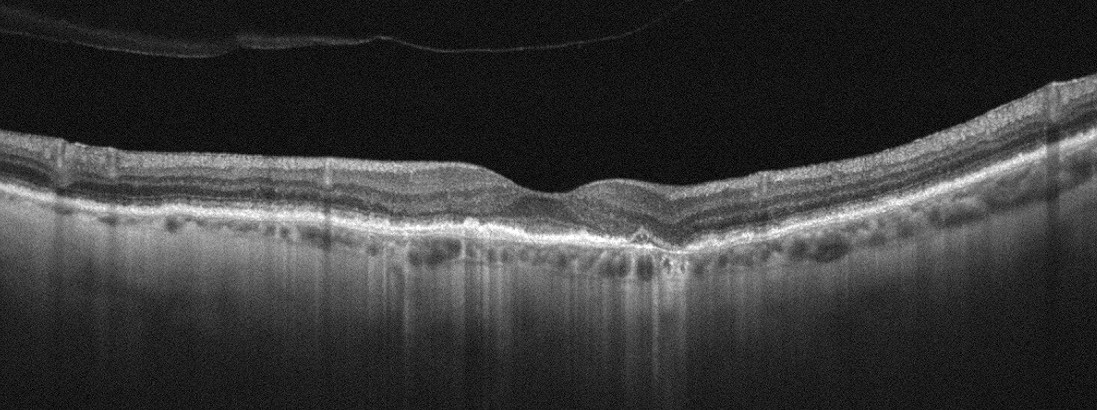
Acquired on an Optovue Avanti RTVue XR · fovea-centered · retinal OCT cross-section.
This B-scan demonstrates age-related macular degeneration.